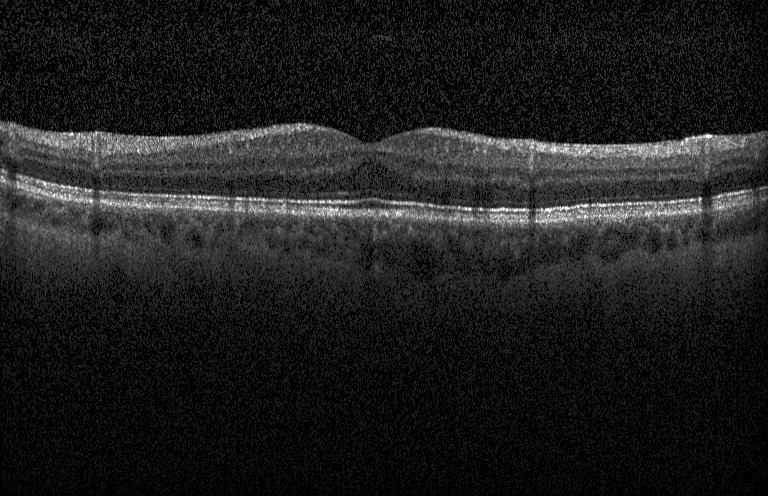

Spectral-domain OCT B-scan: no evidence of CNV, DME, or drusen.